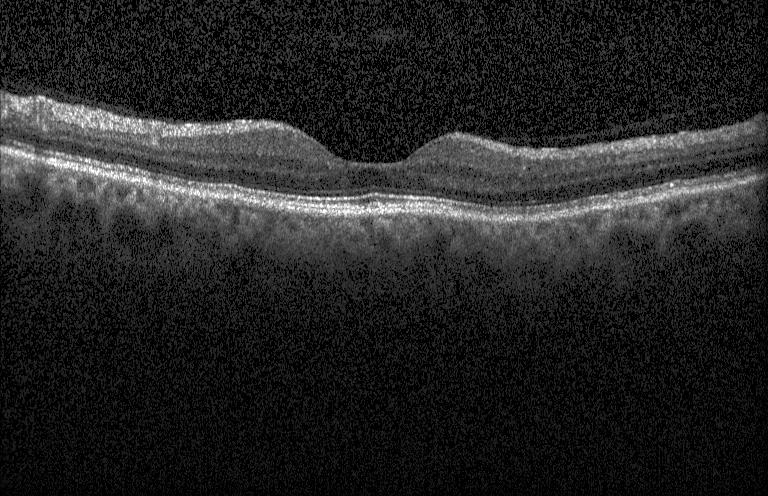

Retinal OCT B-scan · Heidelberg Spectralis OCT system · fovea-centered. Impression: neither choroidal neovascularization, diabetic macular edema, nor drusen.